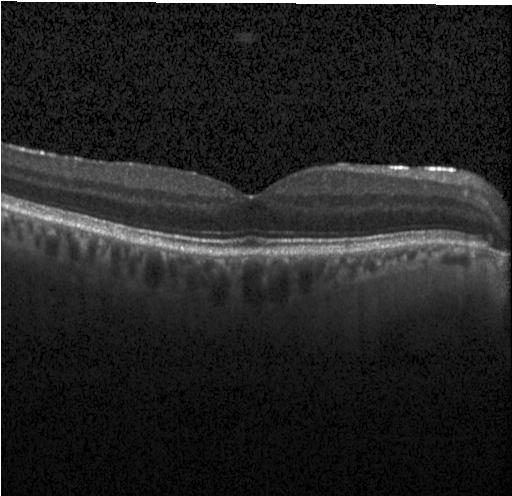

Acquired on a Heidelberg Spectralis. Retinal OCT cross-section. SD-OCT. Neither choroidal neovascularization, diabetic macular edema, nor drusen.